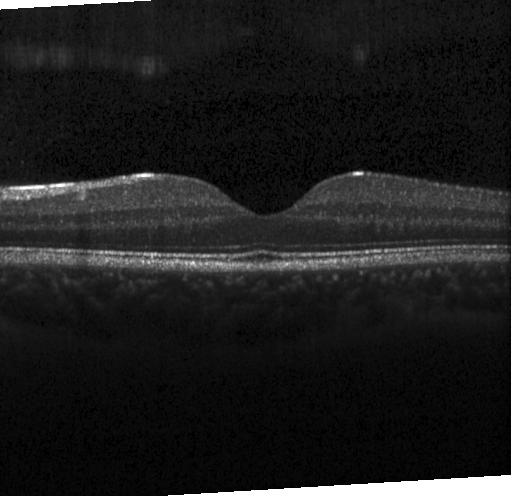 OCT line scan.
This B-scan demonstrates no choroidal neovascularization, no diabetic macular edema, and no drusen.